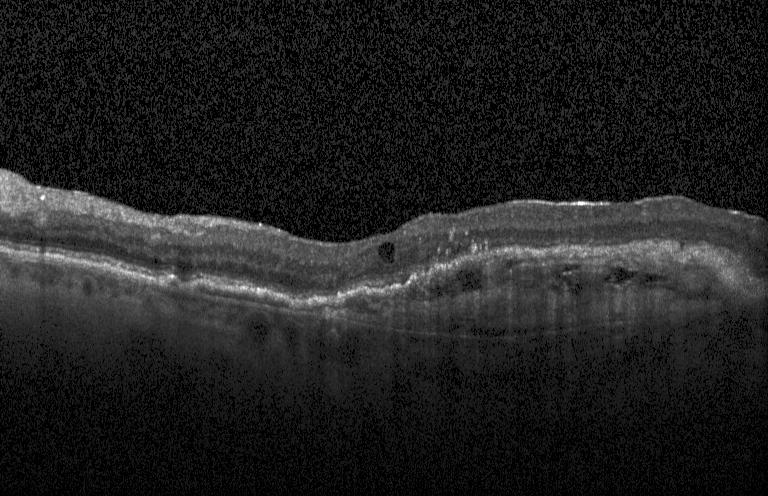 Spectral-domain OCT B-scan: a choroidal neovascular membrane.